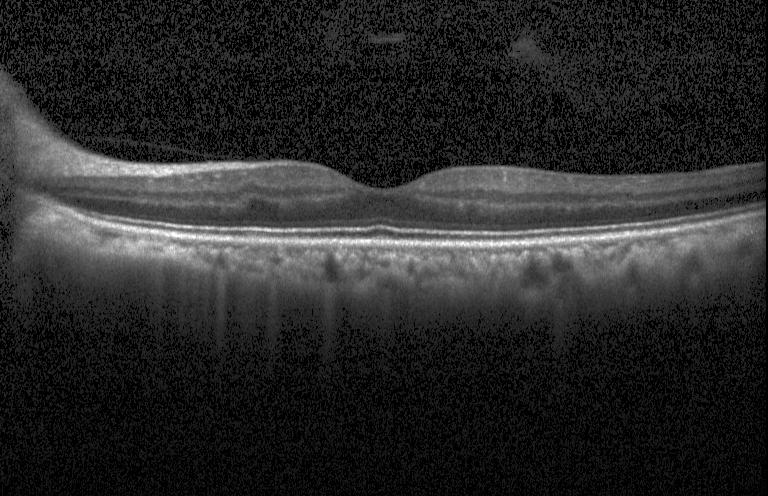

Optical coherence tomography B-scan, centered on the fovea — Macular OCT: no CNV, no DME, and no drusen.